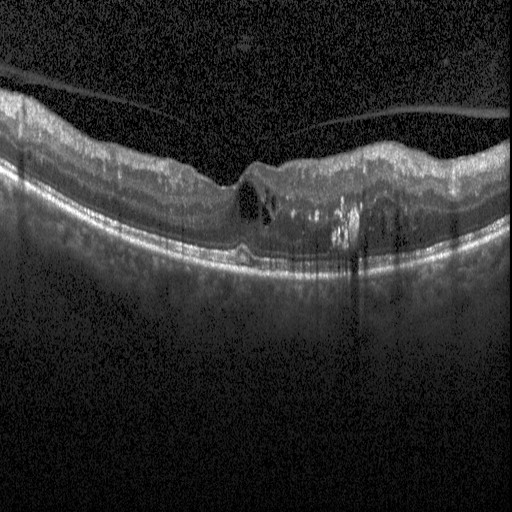
Optical coherence tomography B-scan. DME.